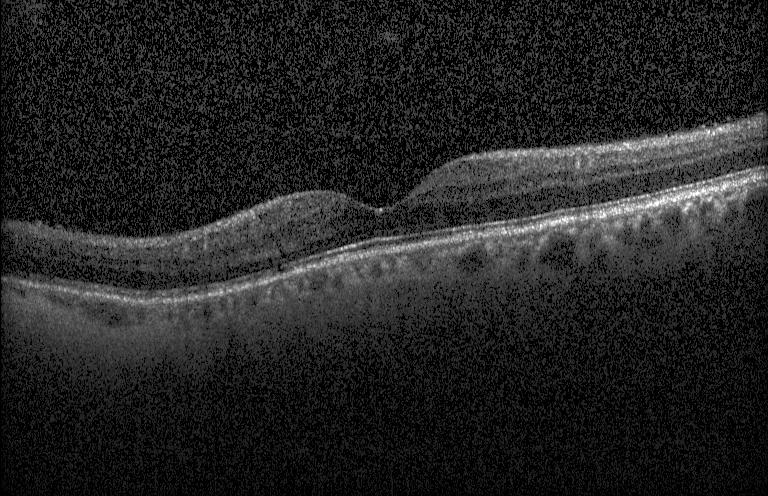

OCT finding: no CNV, no DME, and no drusen.